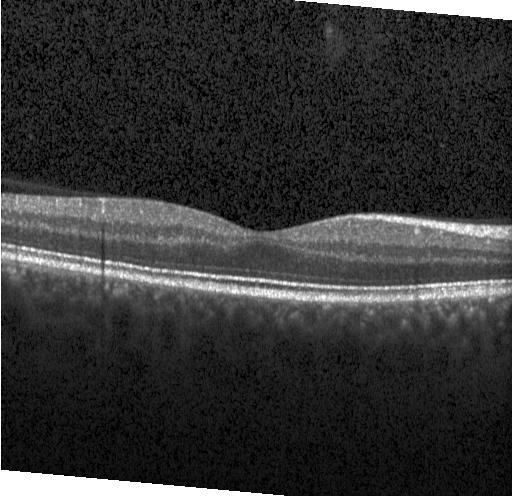

Spectral-domain optical coherence tomography, retinal OCT cross-section, macular scan
Assessment: neither choroidal neovascularization, diabetic macular edema, nor drusen.